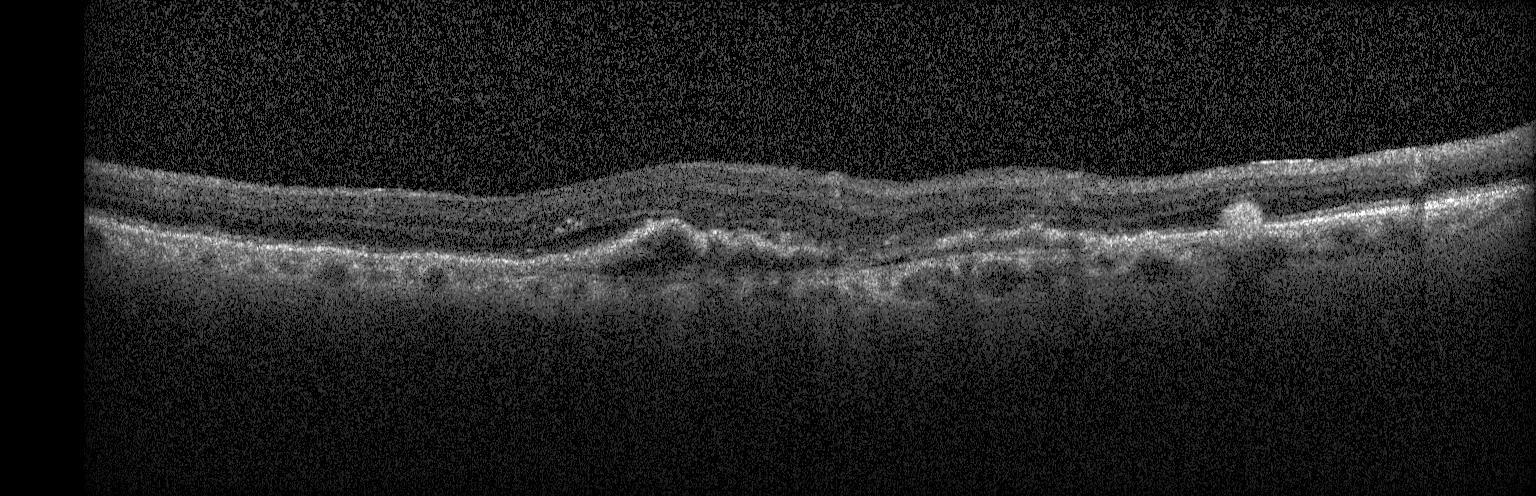
OCT line scan
Assessment: choroidal neovascularization (CNV).